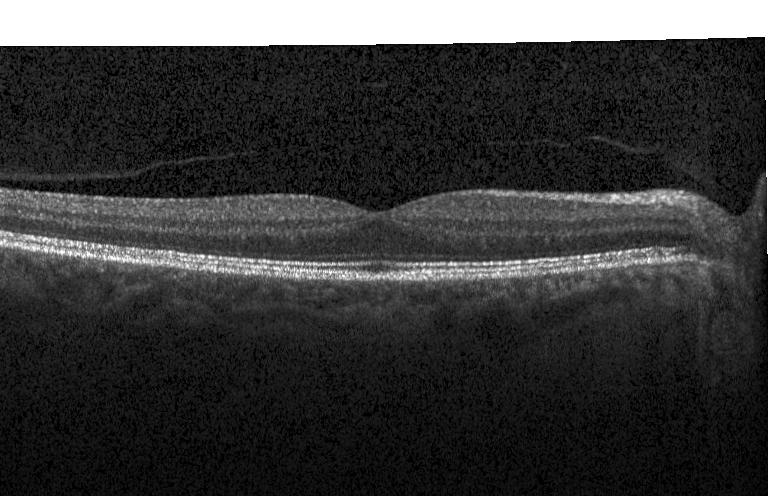

Retinal OCT cross-section; spectral-domain optical coherence tomography
Macular OCT: no evidence of choroidal neovascularization, diabetic macular edema, or drusen.